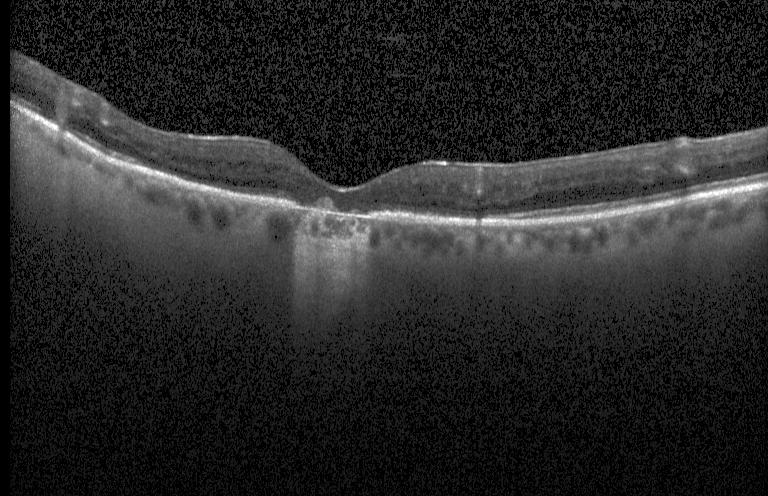 Horizontal scan through the fovea. Instrument: Heidelberg Spectralis. Optical coherence tomography scan. Spectral-domain optical coherence tomography
Choroidal neovascularization.